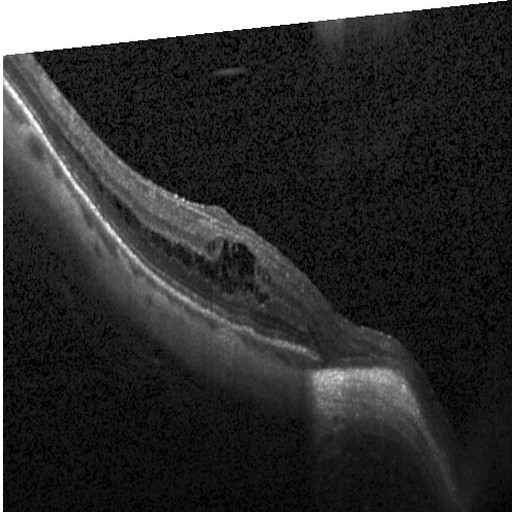 Optical coherence tomography B-scan, SD-OCT, Heidelberg Spectralis.
Diagnosis: diabetic macular edema.